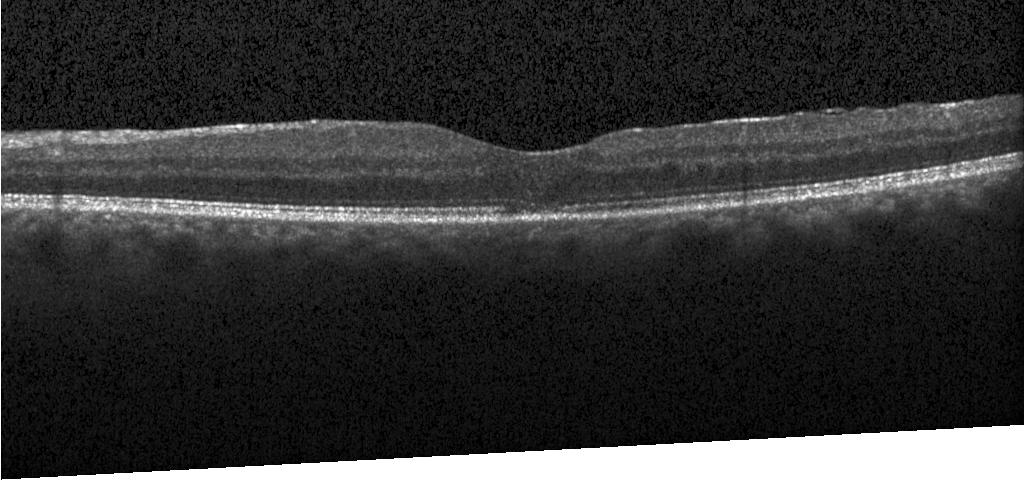 Centered on the fovea; retinal OCT cross-section; spectral-domain OCT
No evidence of choroidal neovascularization, diabetic macular edema, or drusen.